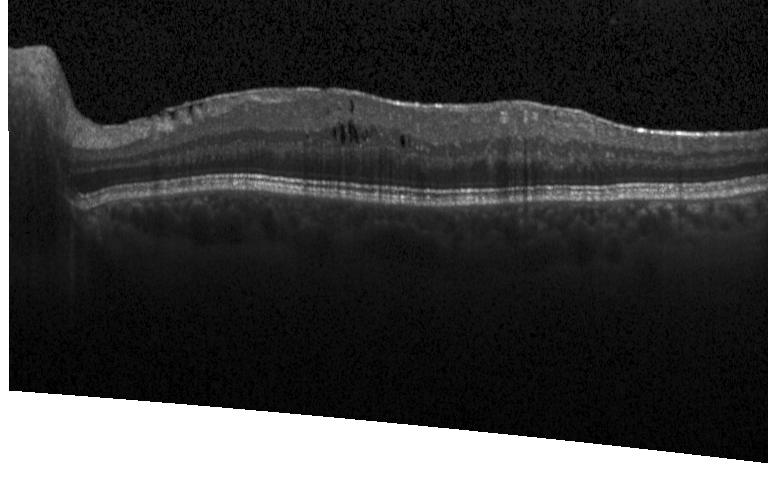
Retinal OCT cross-section · Heidelberg Spectralis OCT system · spectral-domain optical coherence tomography · macular scan. The scan shows DME.